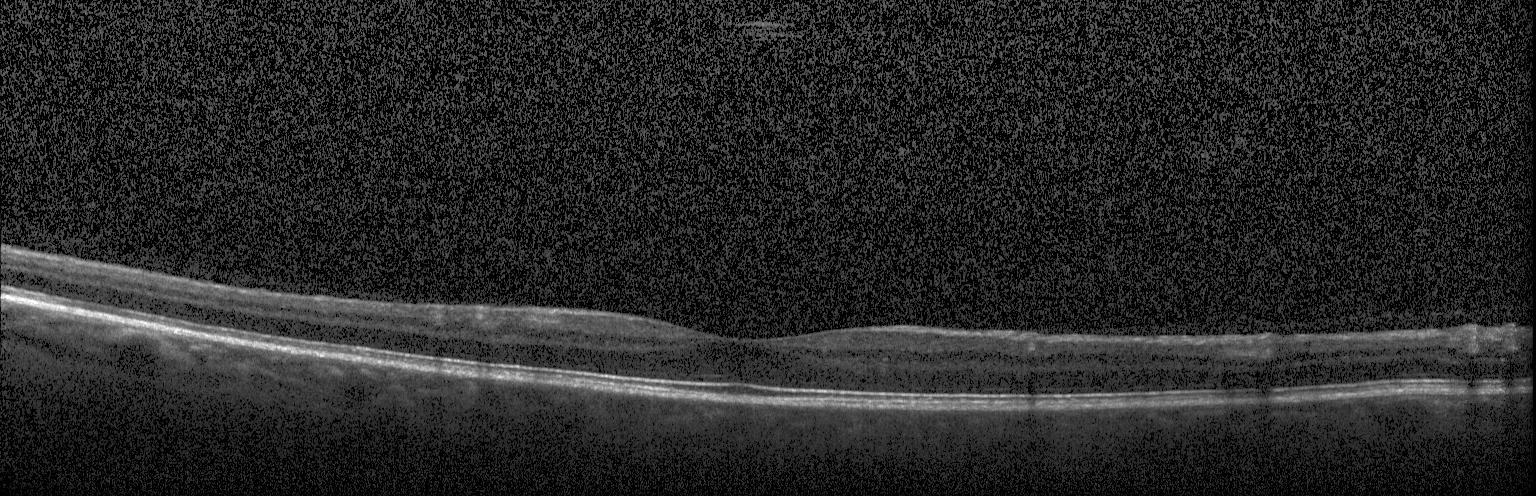

Instrument: Heidelberg Spectralis; through the macula; spectral-domain optical coherence tomography; optical coherence tomography scan — Neither choroidal neovascularization, diabetic macular edema, nor drusen.